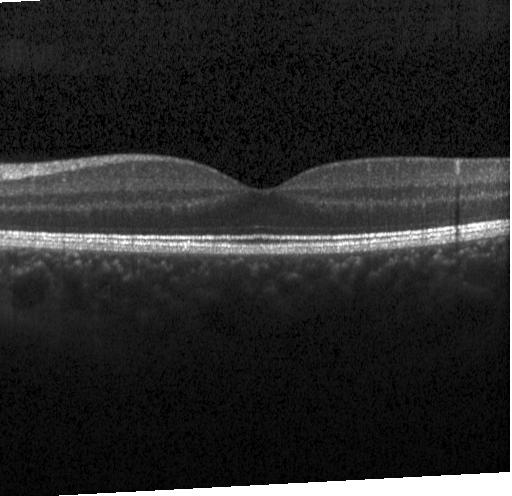 Finding: neither CNV, DME, nor drusen.